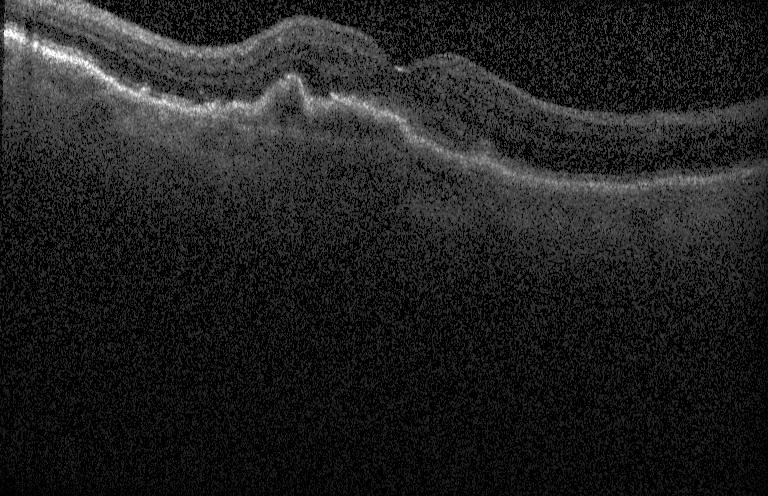 Heidelberg Spectralis, optical coherence tomography B-scan, SD-OCT, centered on the fovea
Diagnosis: a choroidal neovascular membrane.